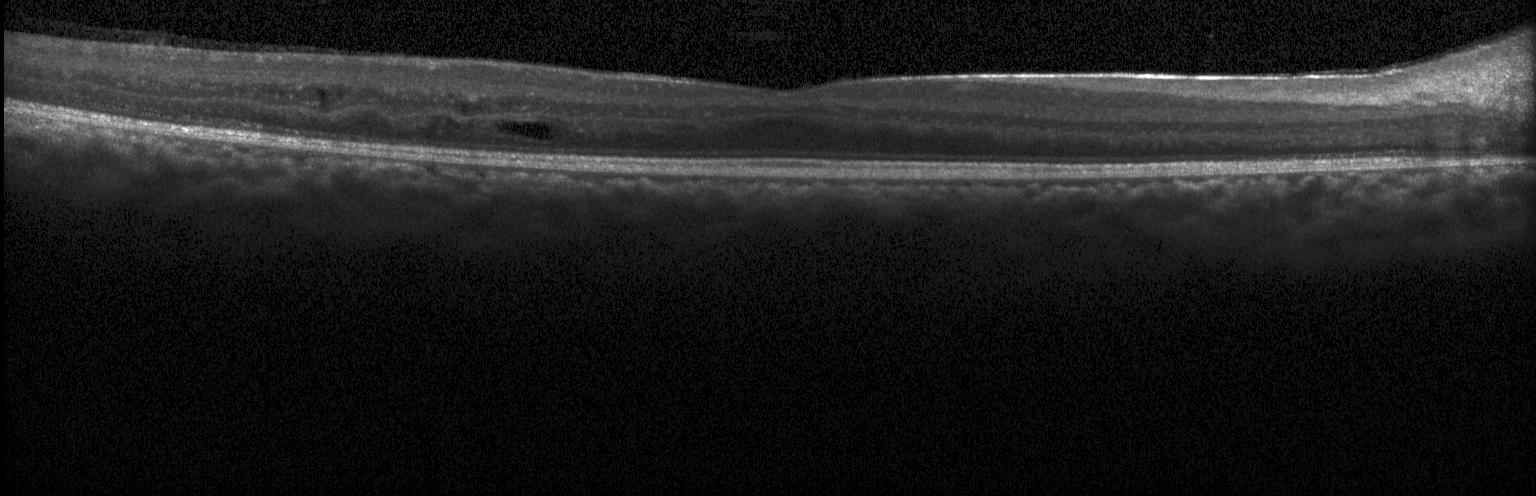
Macular scan. Spectral-domain optical coherence tomography. Heidelberg Spectralis OCT system. Retinal OCT cross-section — Assessment: diabetic macular edema.